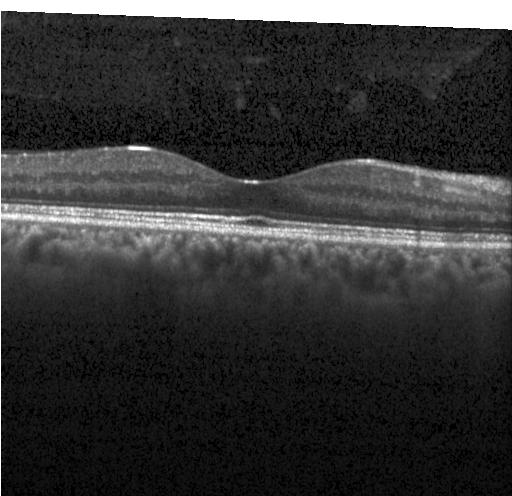

Retinal OCT B-scan.
Finding: neither choroidal neovascularization, diabetic macular edema, nor drusen.